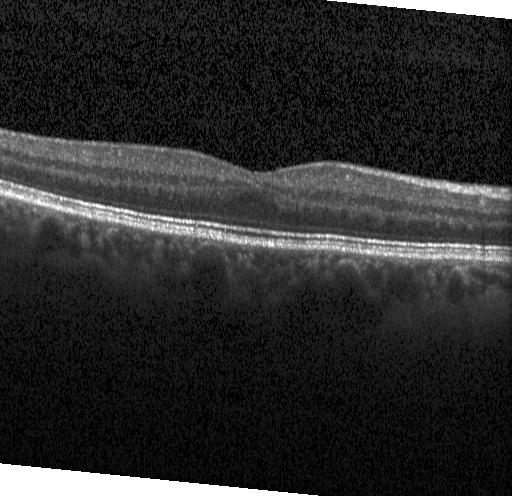
Acquired on a Heidelberg Spectralis, retinal OCT cross-section. No choroidal neovascularization, diabetic macular edema, or drusen.